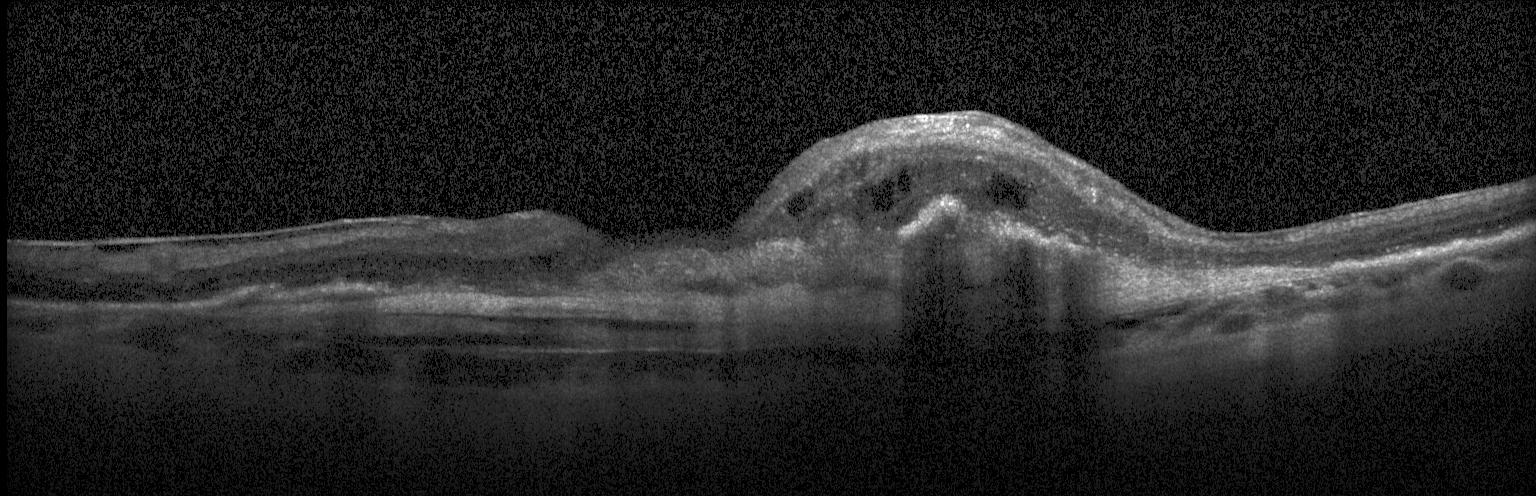

Macular OCT: a choroidal neovascular membrane.